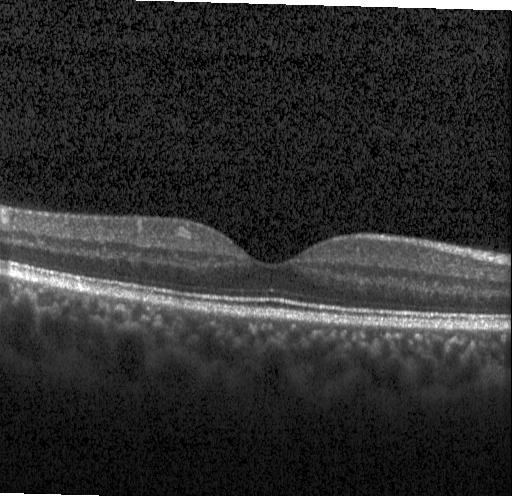 OCT B-scan showing no evidence of choroidal neovascularization, diabetic macular edema, or drusen.